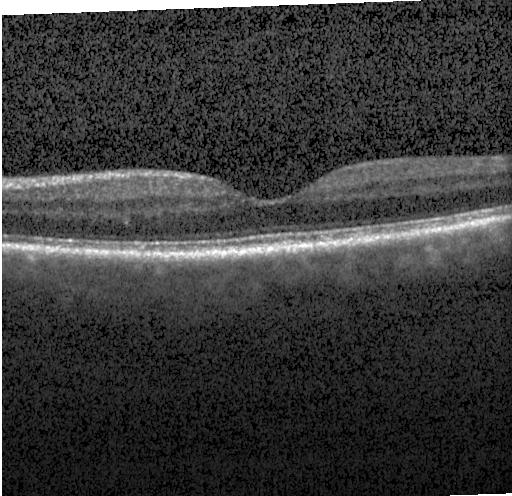 Diagnosis: no CNV, no DME, and no drusen.